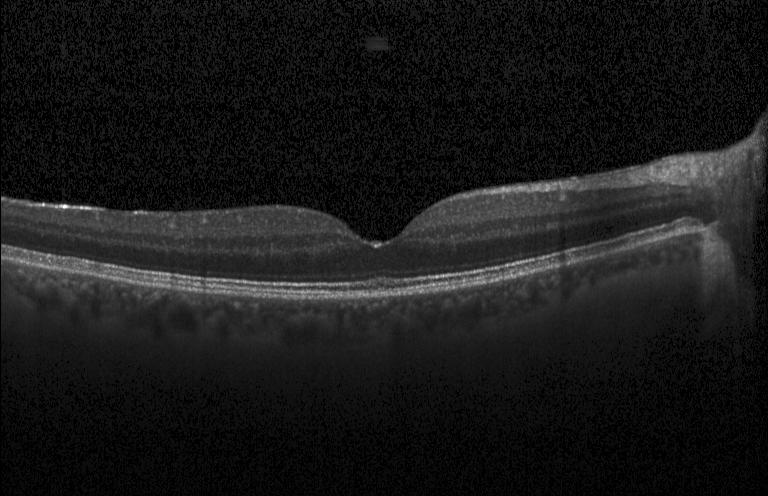 Macular scan; Heidelberg Spectralis; OCT line scan; spectral-domain optical coherence tomography. The scan shows no CNV, DME, or drusen.